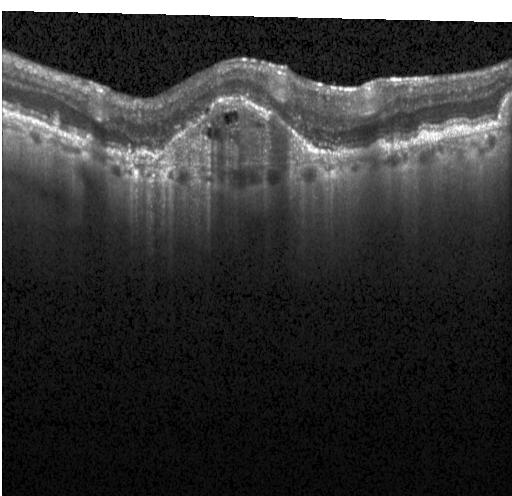

Impression: a choroidal neovascular membrane.